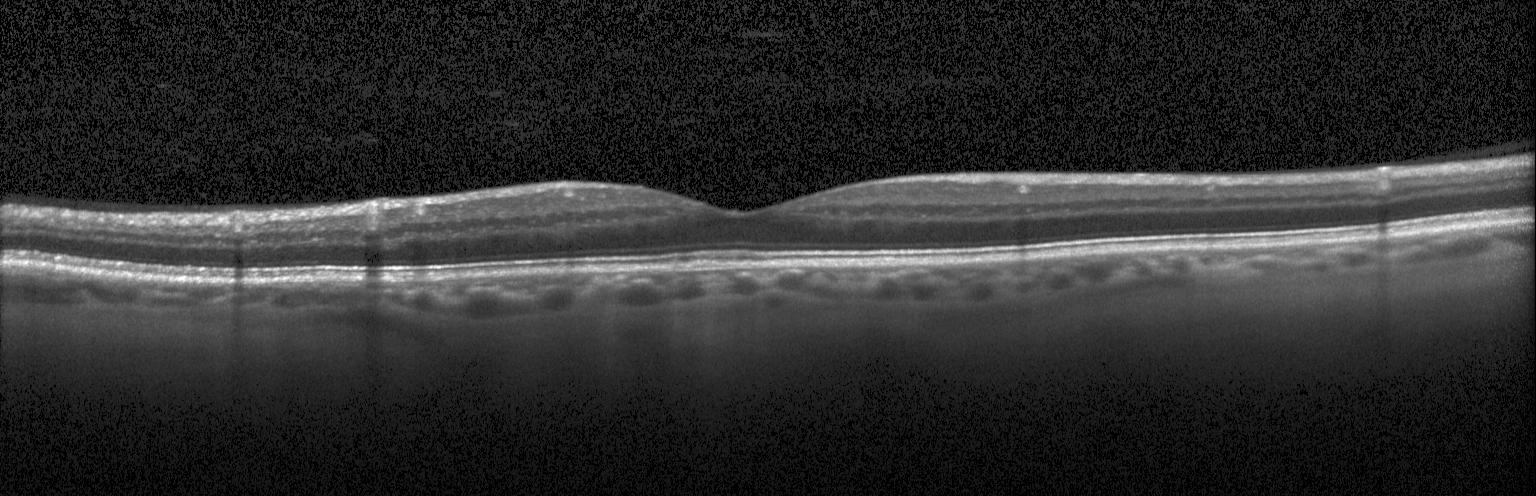

Instrument: Heidelberg Spectralis, retinal OCT B-scan. OCT finding: no choroidal neovascularization, no diabetic macular edema, and no drusen.